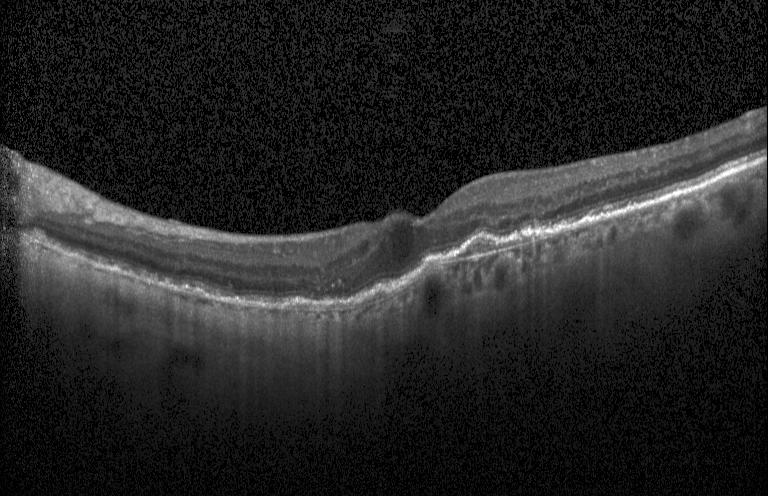
Optical coherence tomography scan — OCT finding: a choroidal neovascular membrane.